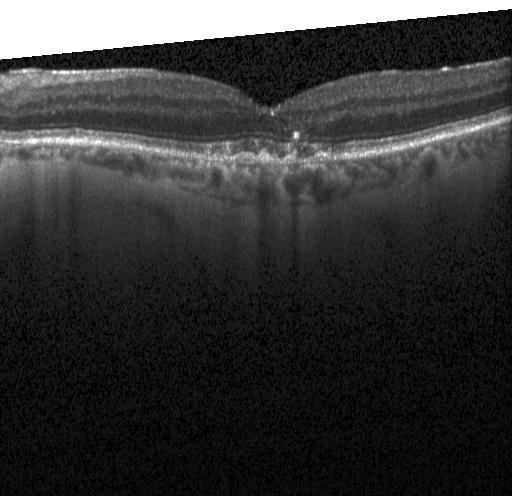 Macular OCT demonstrating a choroidal neovascular membrane.